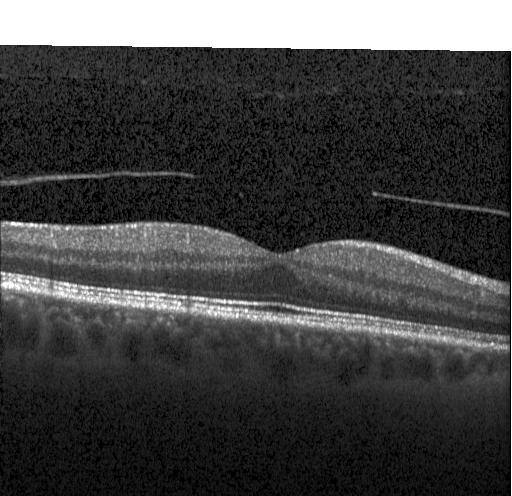
This B-scan demonstrates no choroidal neovascularization, no diabetic macular edema, and no drusen.